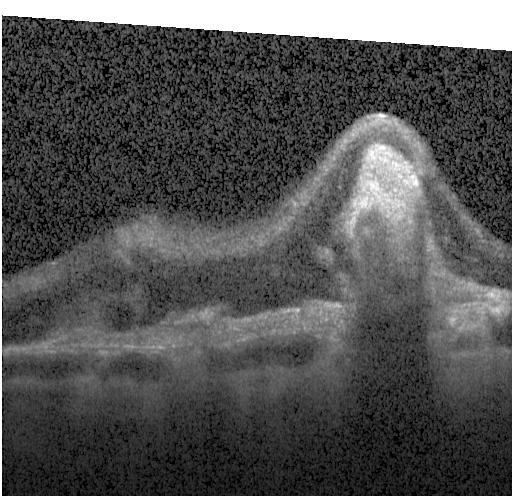

OCT line scan · horizontal scan through the fovea · spectral-domain OCT · instrument: Heidelberg Spectralis — Impression: a choroidal neovascular membrane.